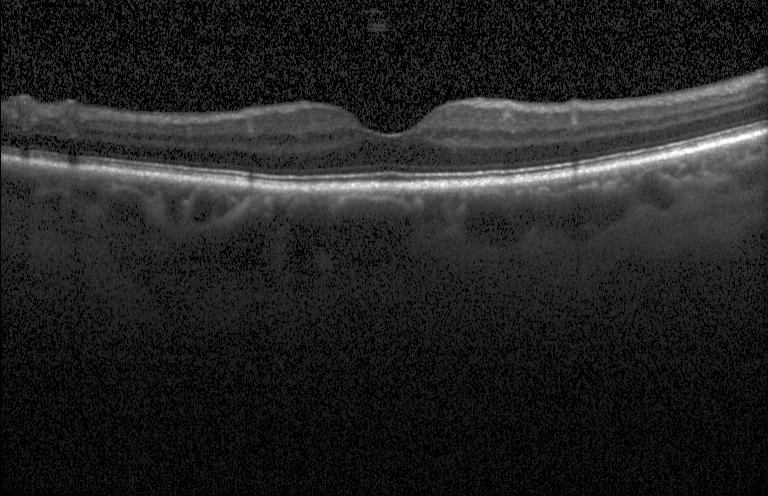
Retinal OCT cross-section — Assessment: no evidence of choroidal neovascularization, diabetic macular edema, or drusen.